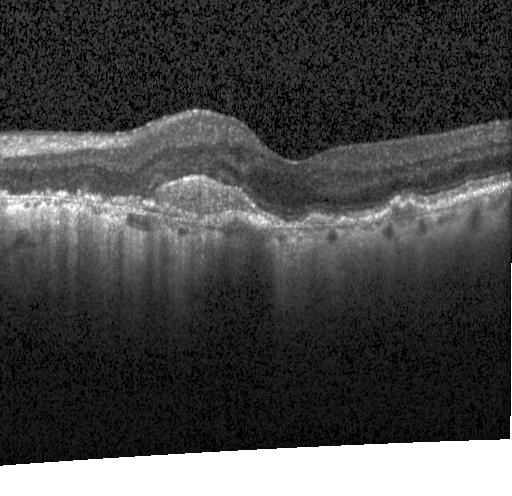
A choroidal neovascular membrane.